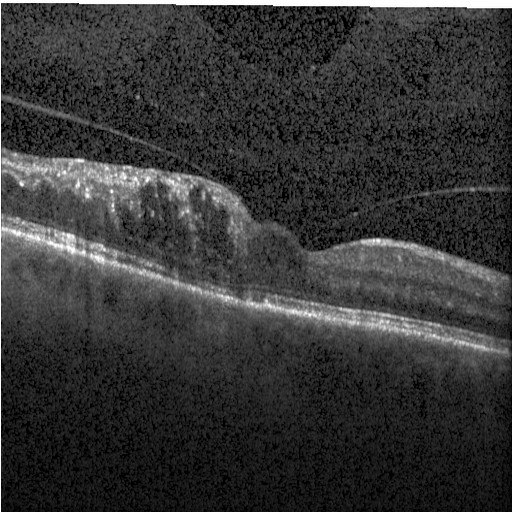

Retinal OCT B-scan. Horizontal scan through the fovea.
Impression: diabetic macular edema.